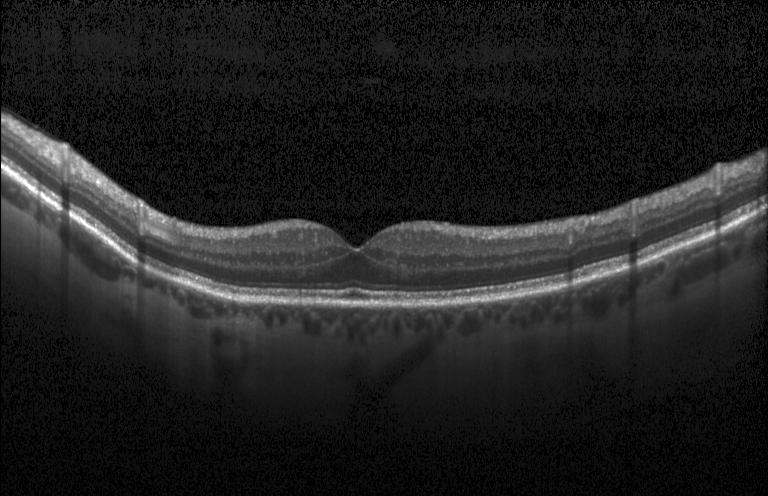

Diagnosis: no CNV, no DME, and no drusen.